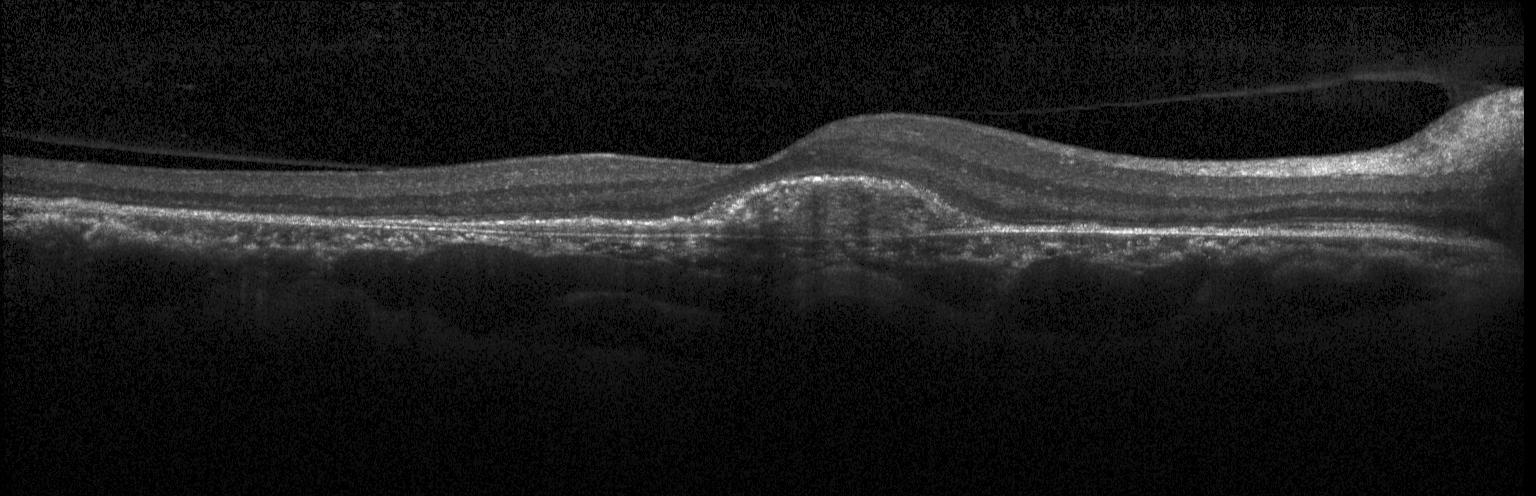
Macular OCT demonstrating a choroidal neovascular membrane.